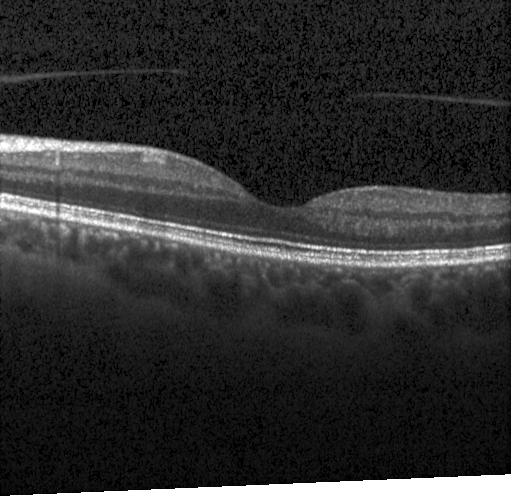 Instrument: Heidelberg Spectralis, optical coherence tomography B-scan, fovea-centered. Diagnosis: no choroidal neovascularization, no diabetic macular edema, and no drusen.